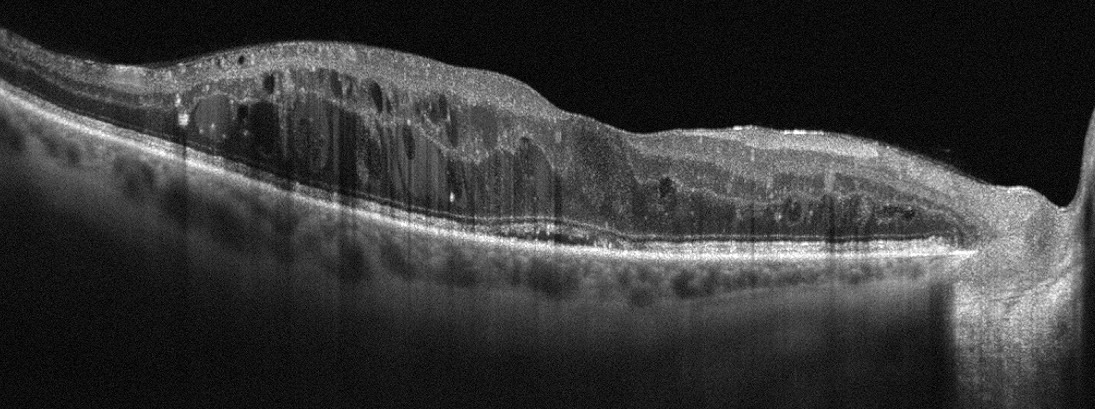 Retinal OCT B-scan. Macular scan. Finding: DME.